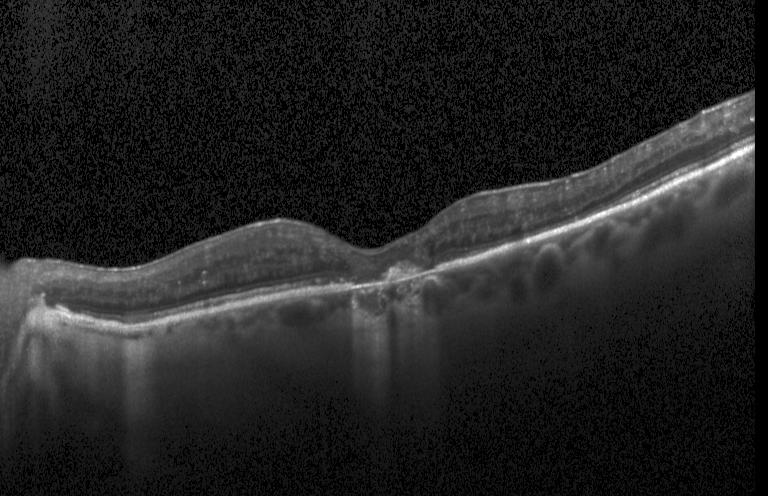 OCT line scan. Impression: a choroidal neovascular membrane.